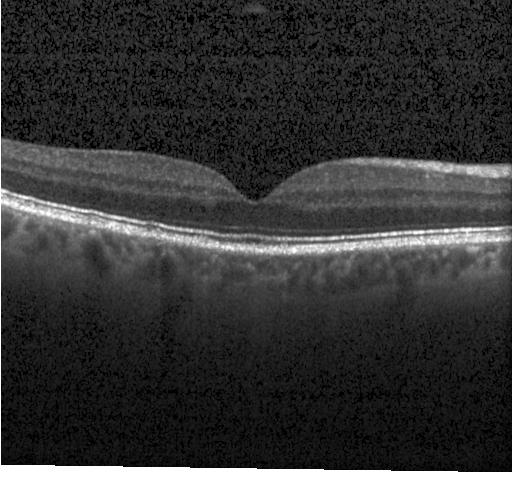 Macular OCT: neither CNV, DME, nor drusen.